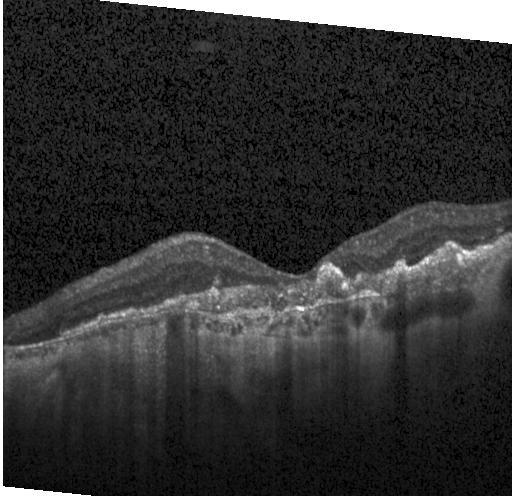
OCT B-scan showing choroidal neovascularization (CNV).